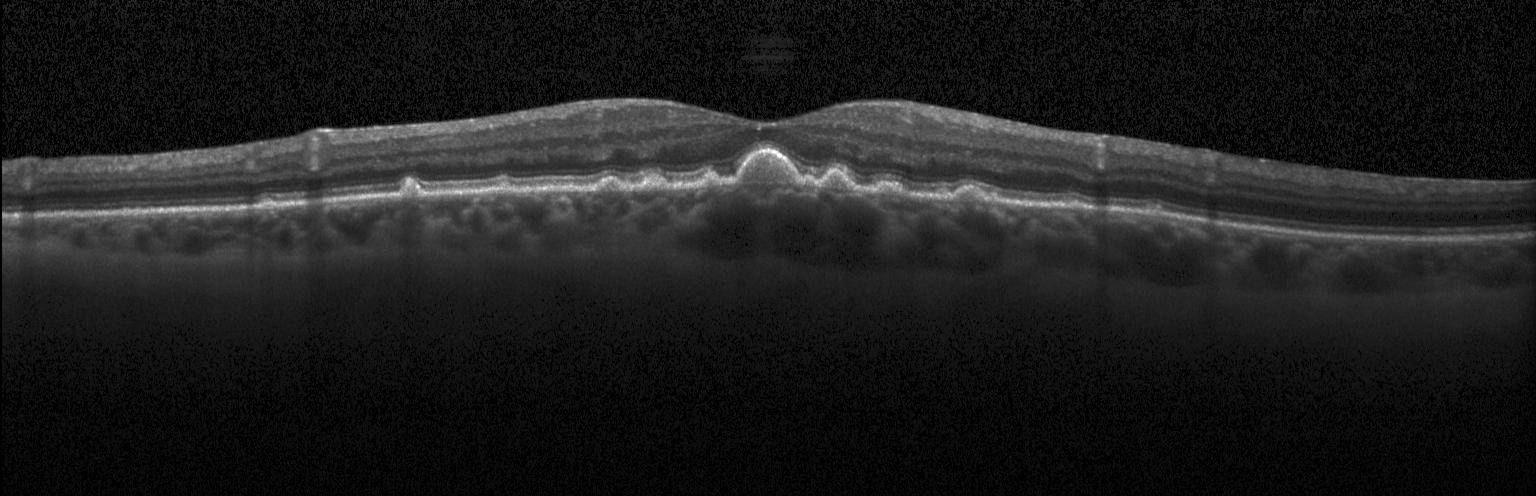

Instrument: Heidelberg Spectralis; retinal OCT cross-section; macular scan; spectral-domain OCT
Multiple drusen.